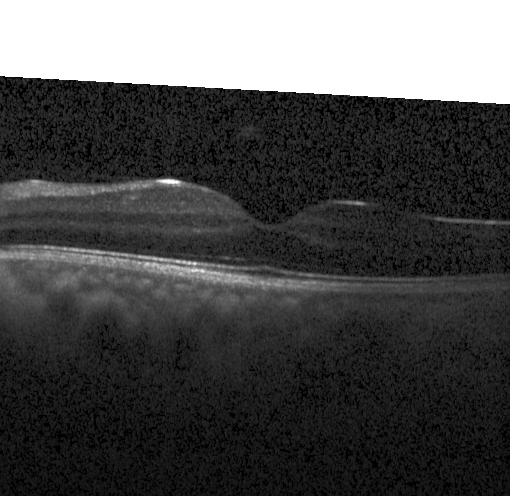 Heidelberg Spectralis OCT system · fovea-centered · spectral-domain optical coherence tomography · OCT B-scan.
Finding: no choroidal neovascularization, no diabetic macular edema, and no drusen.